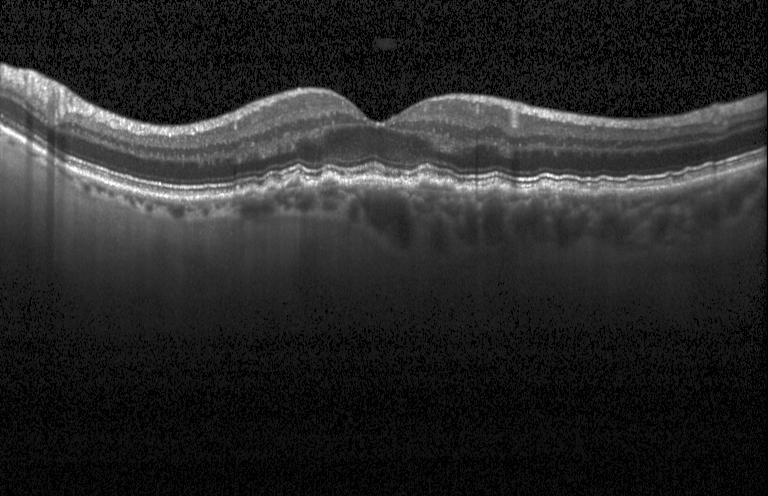 OCT finding: multiple drusen.